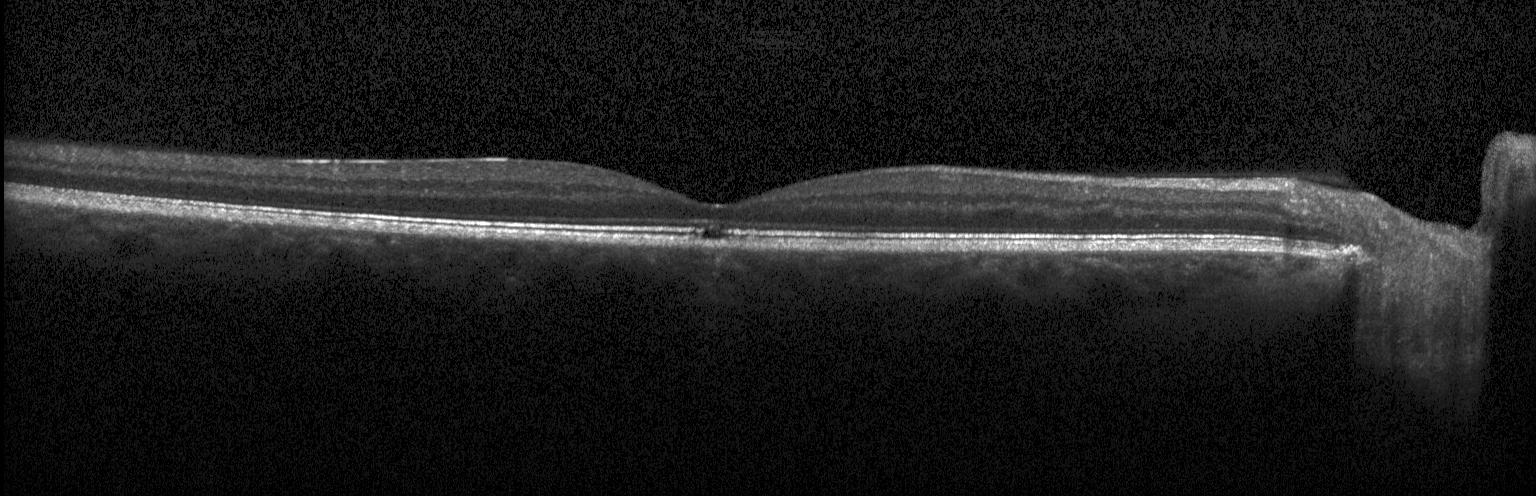 Retinal OCT B-scan
Dx: neither CNV, DME, nor drusen.